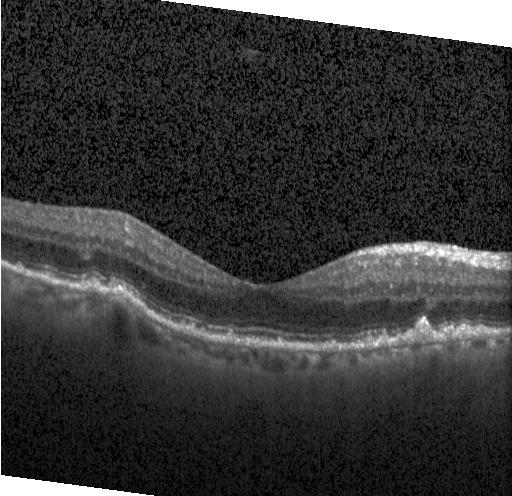 Instrument: Heidelberg Spectralis · through the macula · retinal OCT B-scan · spectral-domain OCT. Diagnosis: drusen.